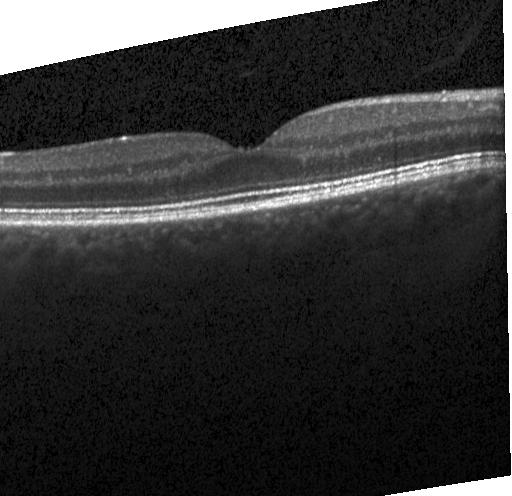 Acquired on a Heidelberg Spectralis · spectral-domain optical coherence tomography · through the macula · optical coherence tomography scan — OCT finding: no evidence of CNV, DME, or drusen.